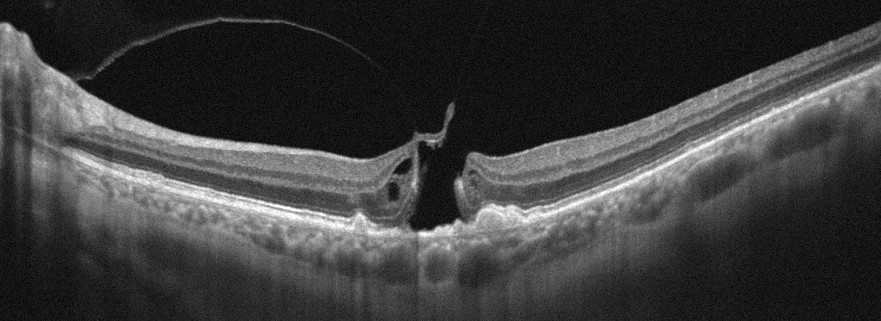 Diagnosis: vitreomacular interface disease (VID).